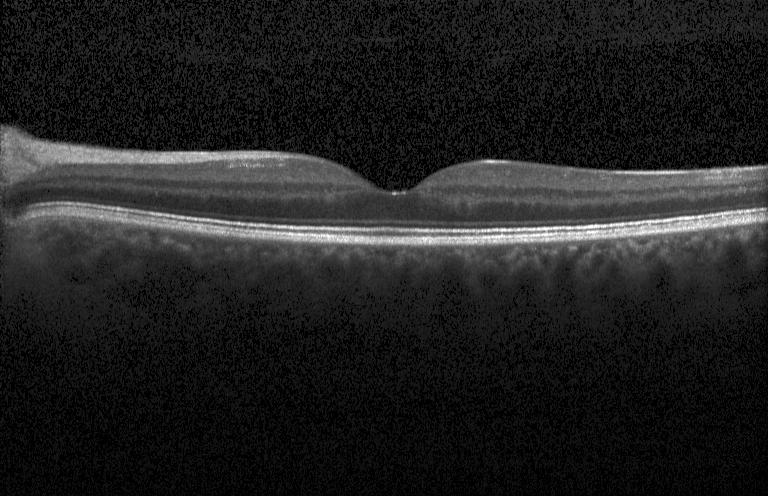
Retinal OCT cross-section — Finding: no choroidal neovascularization, no diabetic macular edema, and no drusen.